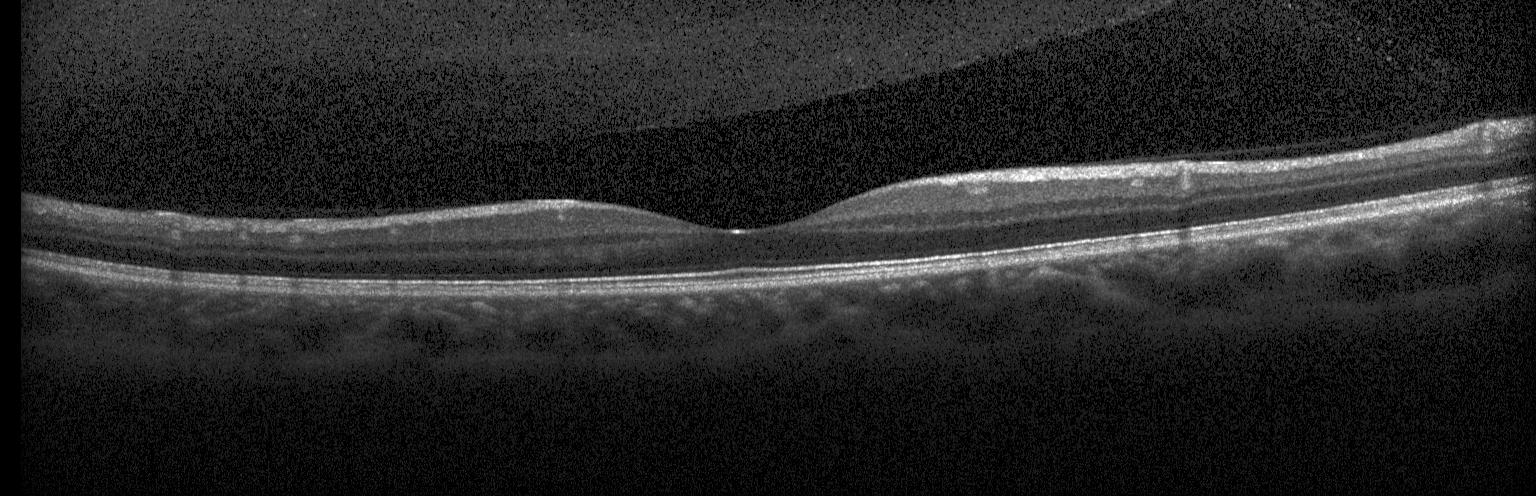

OCT line scan
Assessment: neither choroidal neovascularization, diabetic macular edema, nor drusen.